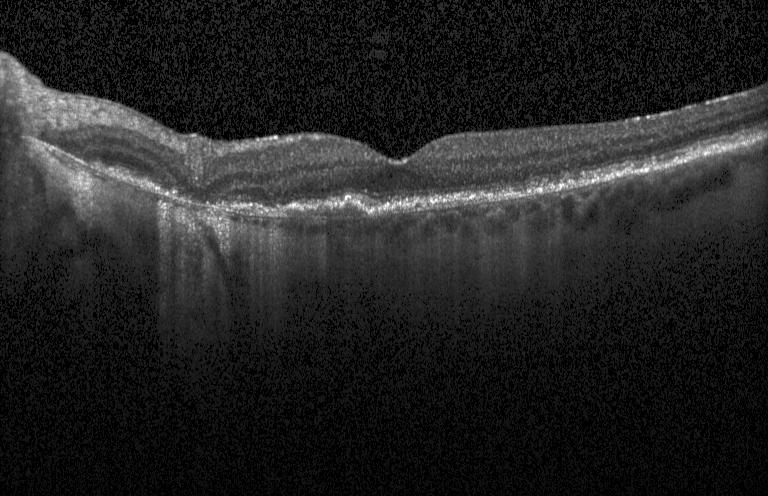
Heidelberg Spectralis OCT system, retinal OCT B-scan
The scan shows CNV.